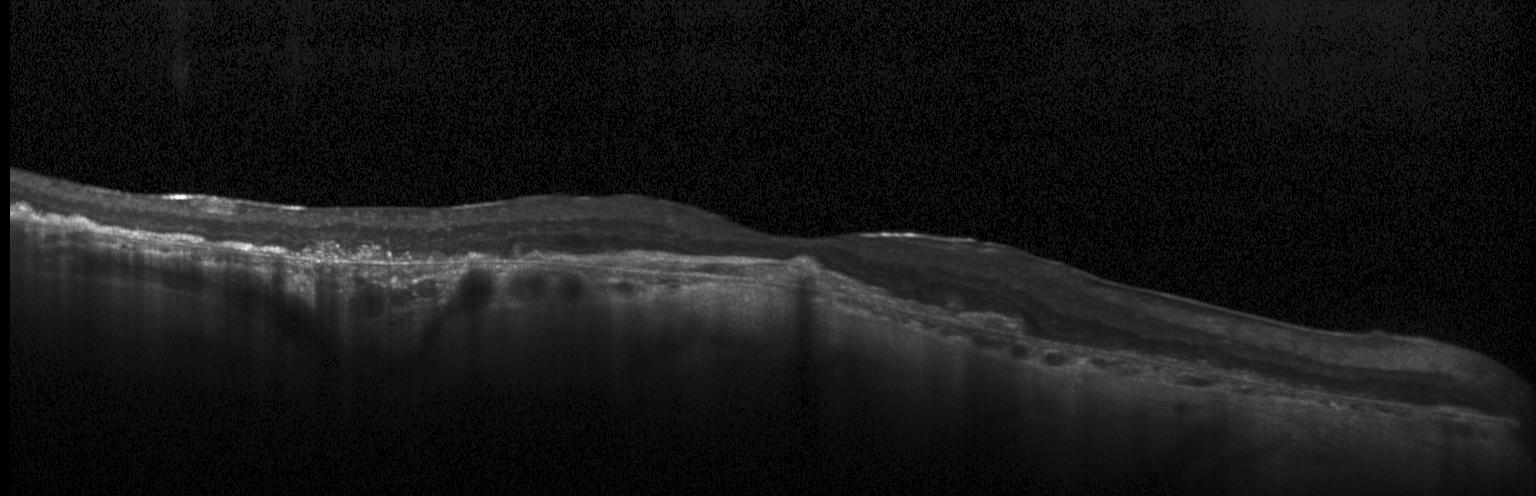

Retinal OCT cross-section showing choroidal neovascularization (CNV).